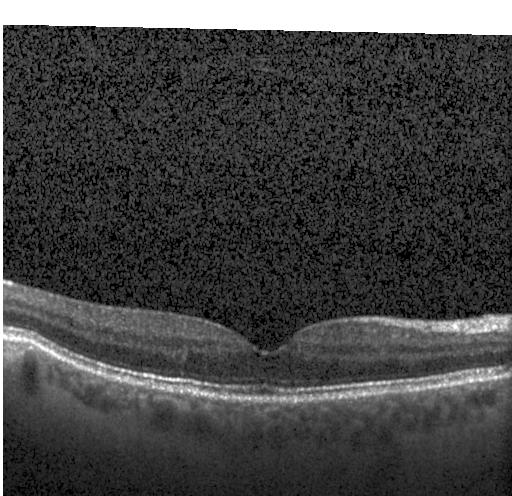 Retinal OCT B-scan.
Diagnosis: no choroidal neovascularization, diabetic macular edema, or drusen.